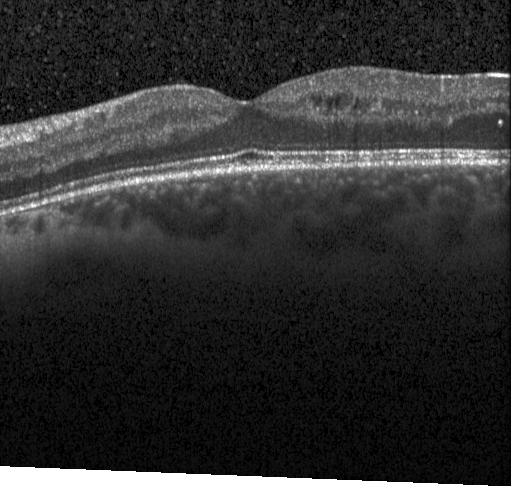 Fovea-centered, retinal OCT B-scan, Heidelberg Spectralis OCT system.
Diagnosis: DME.